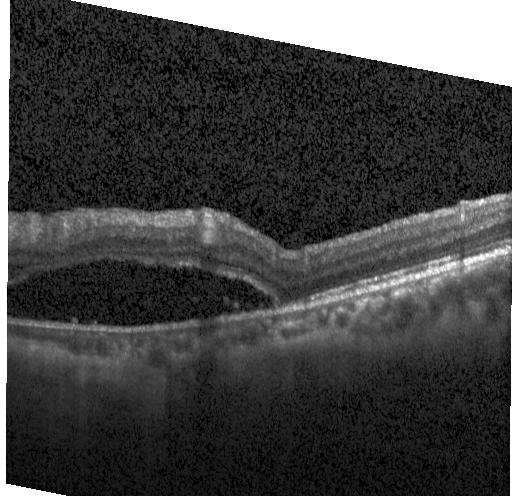

Retinal OCT B-scan — Impression: choroidal neovascularization (CNV).